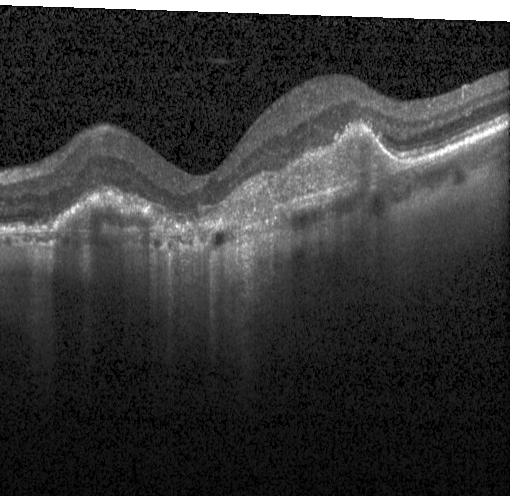
OCT B-scan
Diagnosis: a choroidal neovascular membrane.